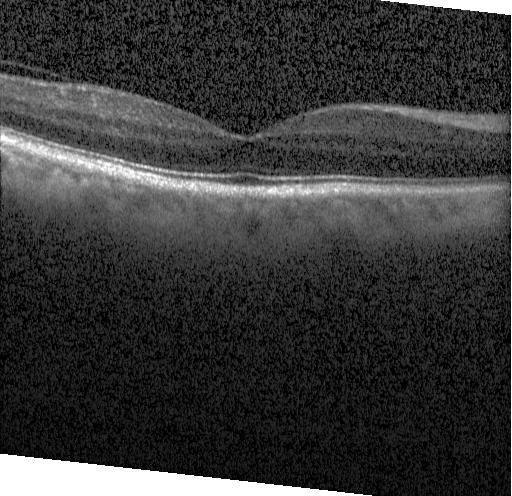 Horizontal scan through the fovea. Instrument: Heidelberg Spectralis. OCT B-scan. Finding: neither choroidal neovascularization, diabetic macular edema, nor drusen.